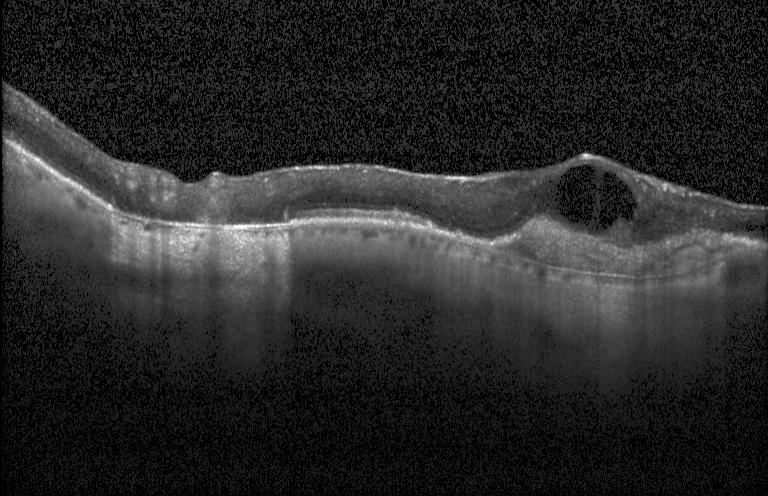

Spectral-domain OCT; macular scan; acquired on a Heidelberg Spectralis; retinal OCT B-scan — Impression: CNV.